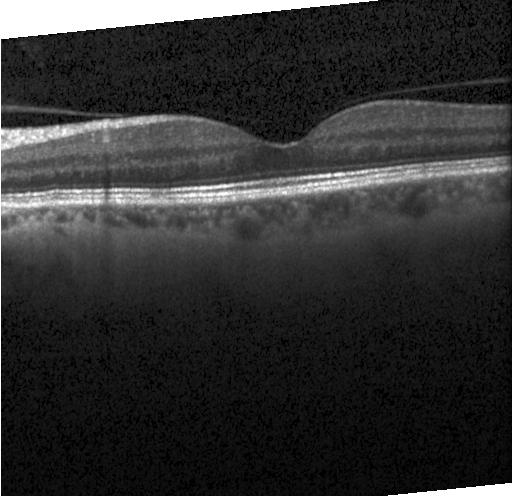

Assessment: no evidence of CNV, DME, or drusen.